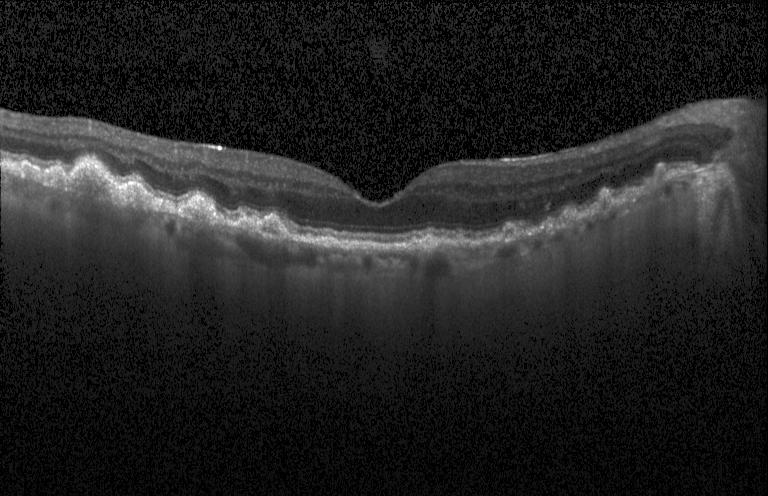

Drusen.